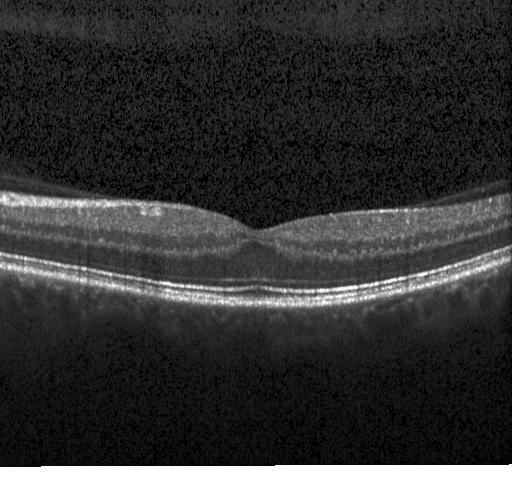

Spectral-domain OCT. Acquired on a Heidelberg Spectralis. Macular scan. Retinal OCT cross-section
Diagnosis: neither CNV, DME, nor drusen.